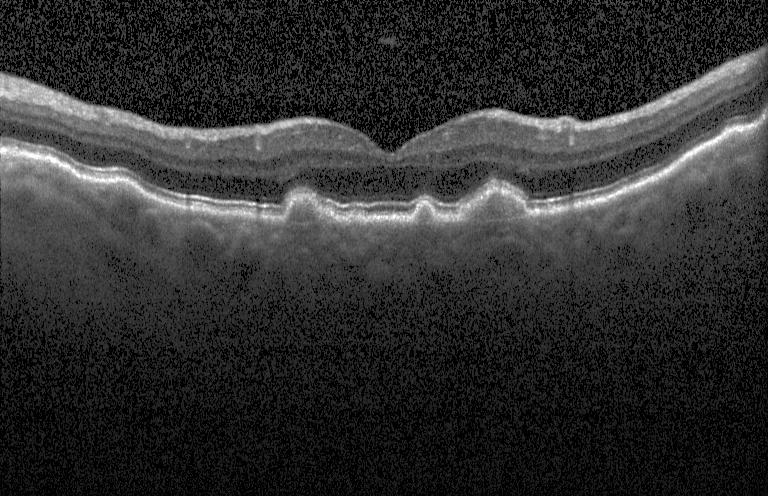 Retinal OCT cross-section; Heidelberg Spectralis; spectral-domain OCT; fovea-centered
Finding: drusen.